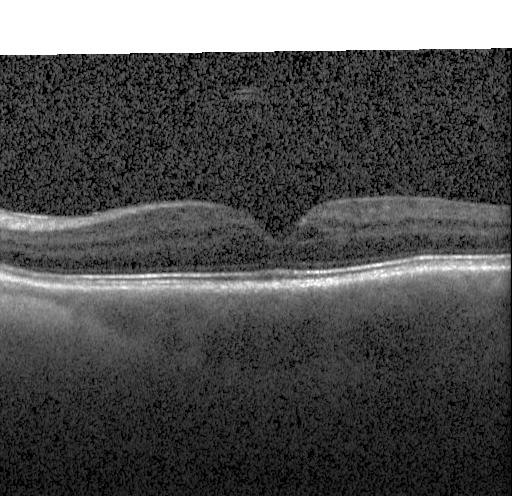 The scan shows diabetic macular edema (DME).